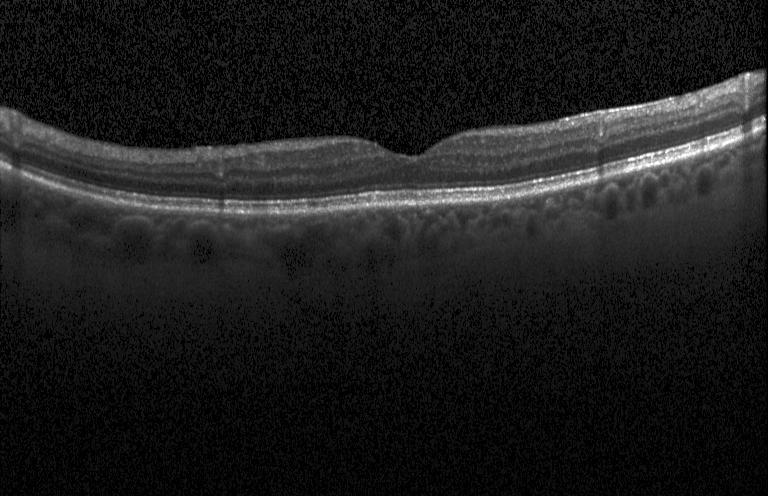 Diagnosis: no choroidal neovascularization, diabetic macular edema, or drusen.